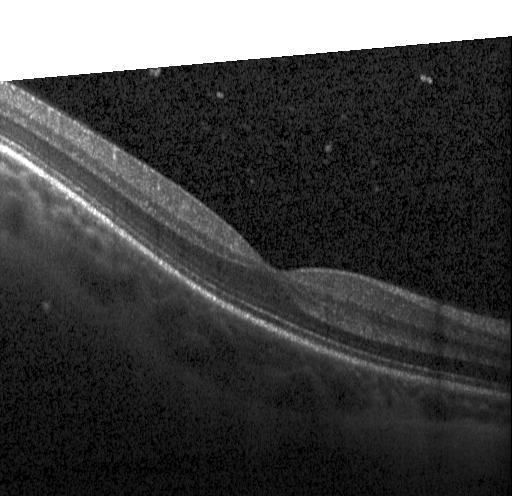
Heidelberg Spectralis. SD-OCT. Optical coherence tomography scan. Finding: no CNV, DME, or drusen.